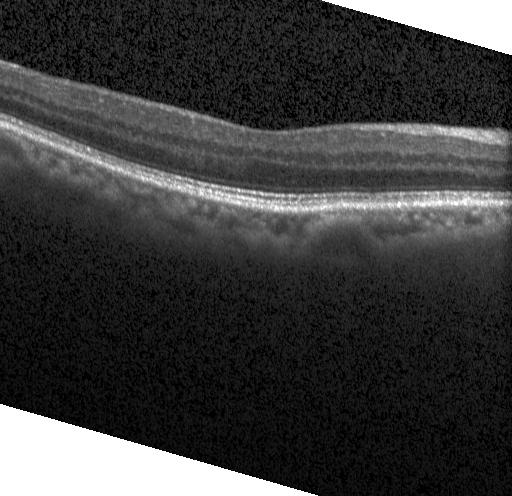 The scan shows no evidence of CNV, DME, or drusen.